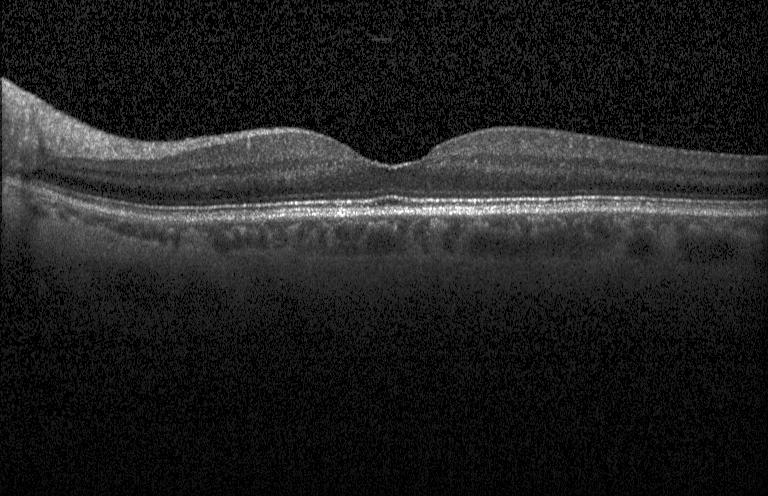
Heidelberg Spectralis, centered on the fovea, OCT line scan, spectral-domain OCT. Assessment: neither CNV, DME, nor drusen.